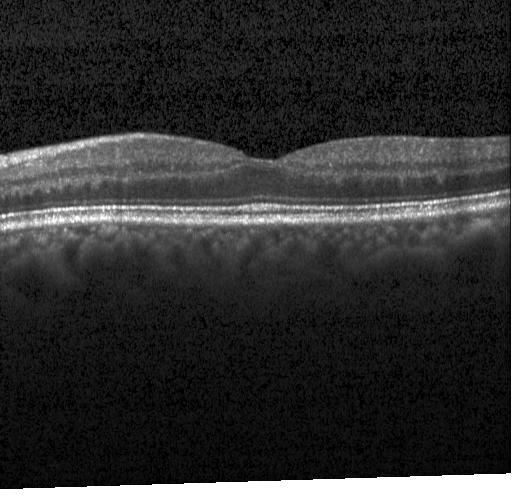
Through the macula; instrument: Heidelberg Spectralis; OCT B-scan; SD-OCT — Assessment: no choroidal neovascularization, no diabetic macular edema, and no drusen.